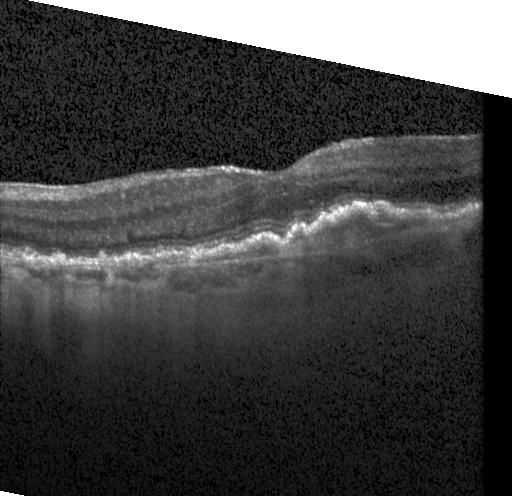 Spectral-domain OCT · horizontal scan through the fovea · Heidelberg Spectralis · optical coherence tomography B-scan
Finding: choroidal neovascularization (CNV).